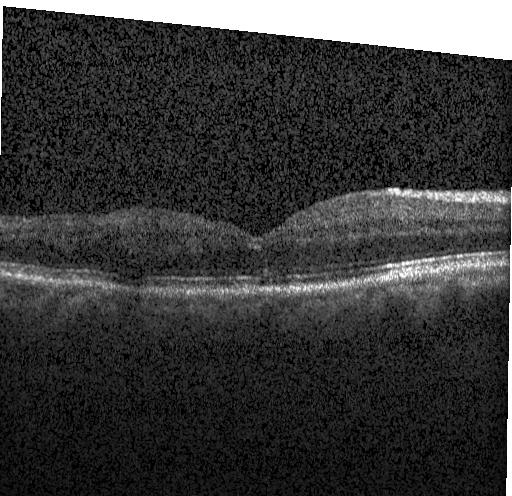

Macular OCT demonstrating no choroidal neovascularization, no diabetic macular edema, and no drusen.